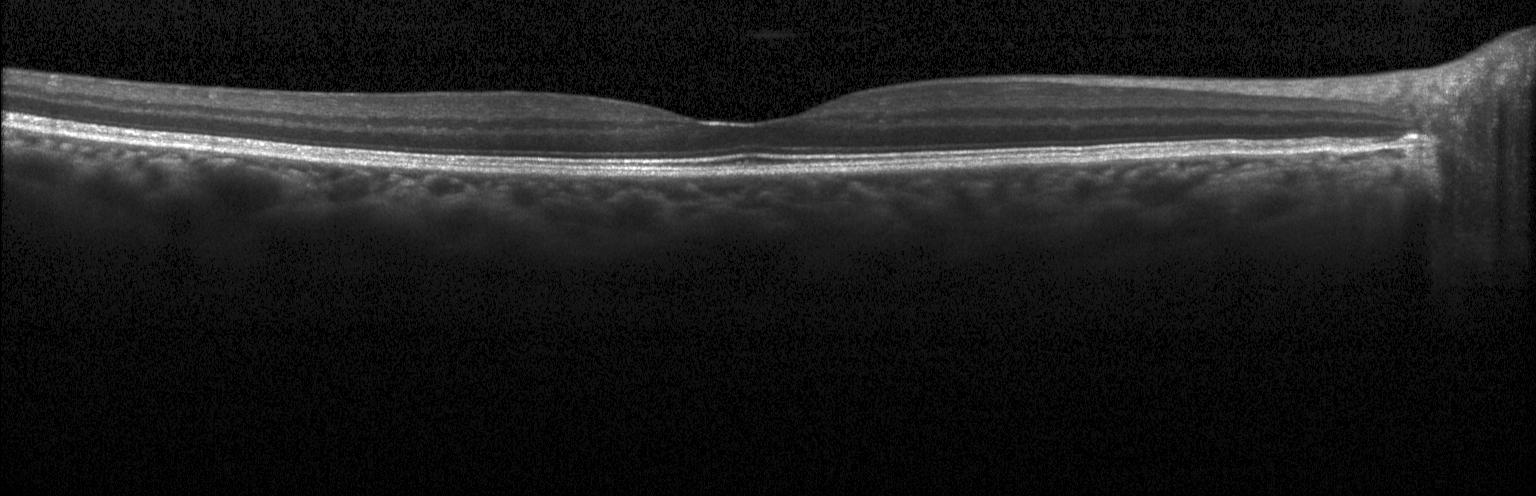 Retinal OCT B-scan.
Finding: neither choroidal neovascularization, diabetic macular edema, nor drusen.